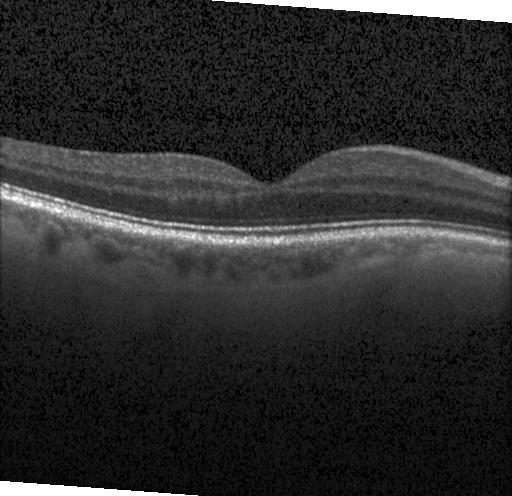
Retinal OCT cross-section.
Impression: no choroidal neovascularization, diabetic macular edema, or drusen.